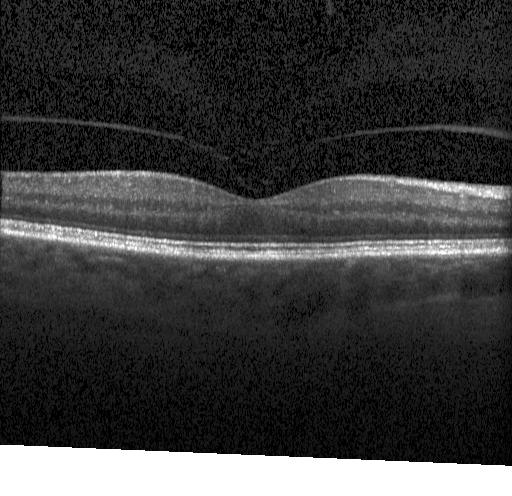
Optical coherence tomography B-scan.
Finding: no choroidal neovascularization, no diabetic macular edema, and no drusen.